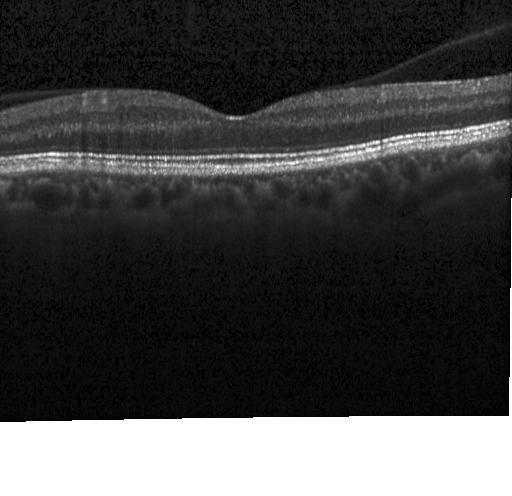

Finding: no evidence of choroidal neovascularization, diabetic macular edema, or drusen.